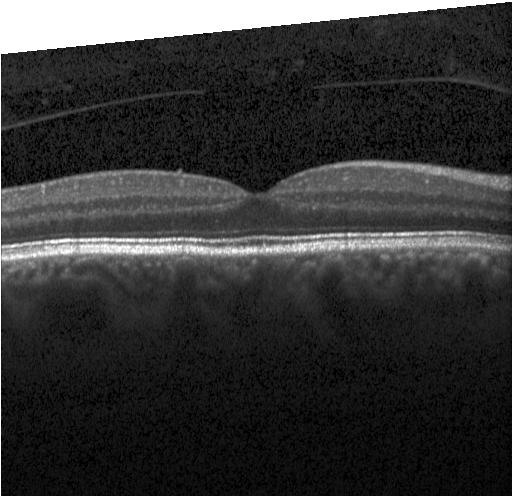
Fovea-centered · retinal OCT B-scan
Finding: no evidence of choroidal neovascularization, diabetic macular edema, or drusen.